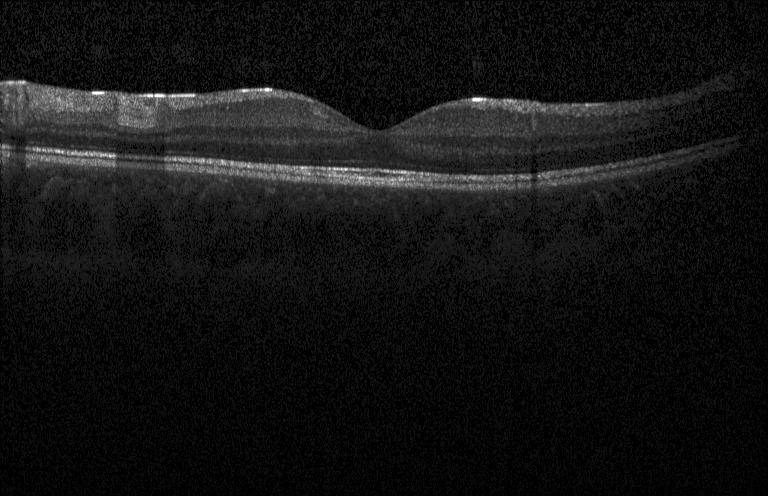
Impression: neither CNV, DME, nor drusen.